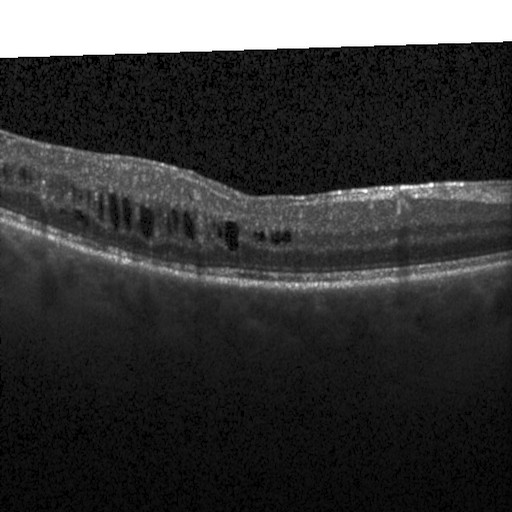

Retinal OCT cross-section showing diabetic macular edema (DME).